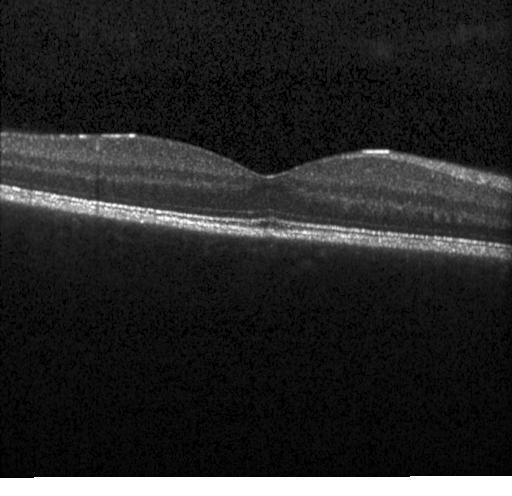
Finding: no CNV, no DME, and no drusen.